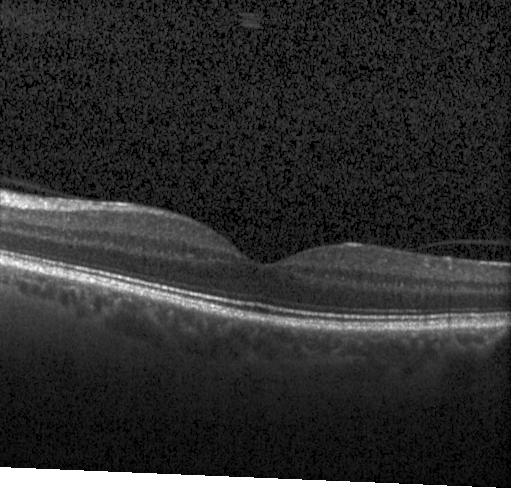

Retinal OCT cross-section showing no evidence of choroidal neovascularization, diabetic macular edema, or drusen.